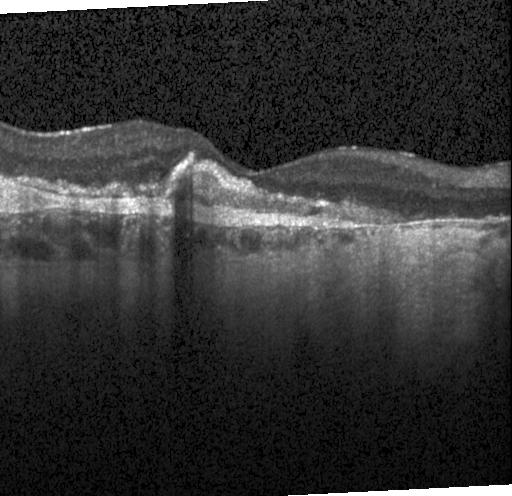 OCT B-scan — Macular OCT: choroidal neovascularization.